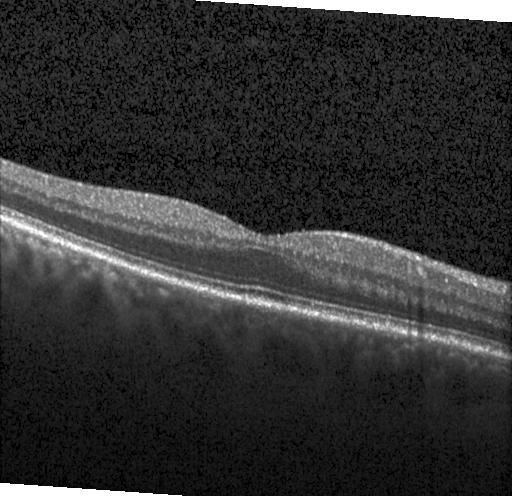

OCT B-scan — No evidence of choroidal neovascularization, diabetic macular edema, or drusen.